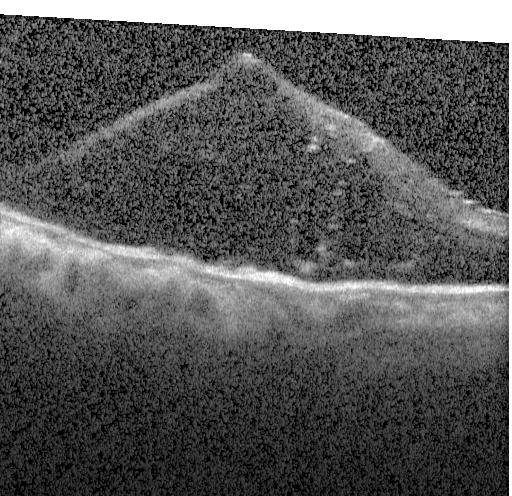
Spectral-domain optical coherence tomography. Retinal OCT cross-section.
Assessment: DME.